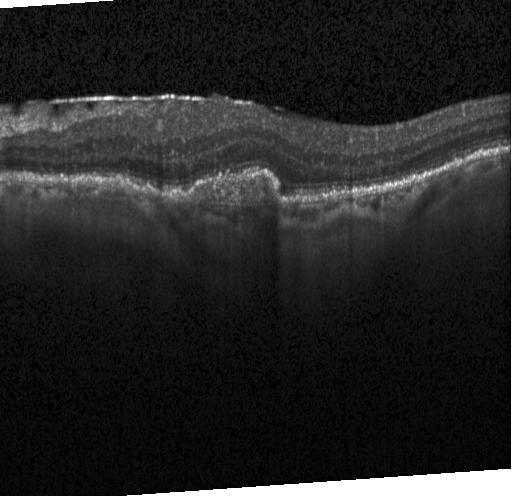

Optical coherence tomography scan. Dx: a choroidal neovascular membrane.